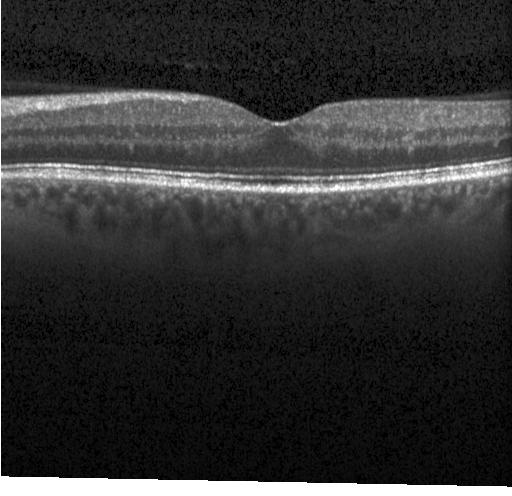 Spectral-domain optical coherence tomography, horizontal scan through the fovea, Heidelberg Spectralis OCT system, OCT line scan.
Assessment: no evidence of CNV, DME, or drusen.